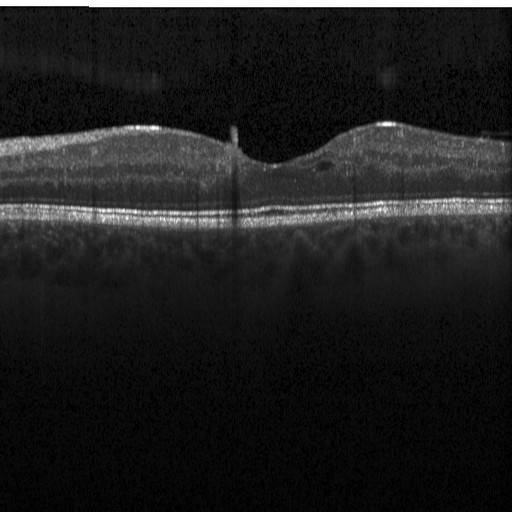
Optical coherence tomography B-scan.
Macular OCT: DME.